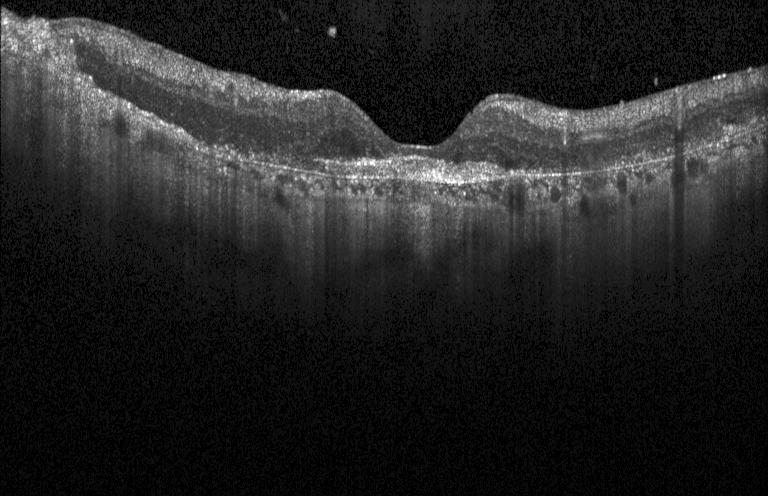 OCT line scan.
Dx: CNV.